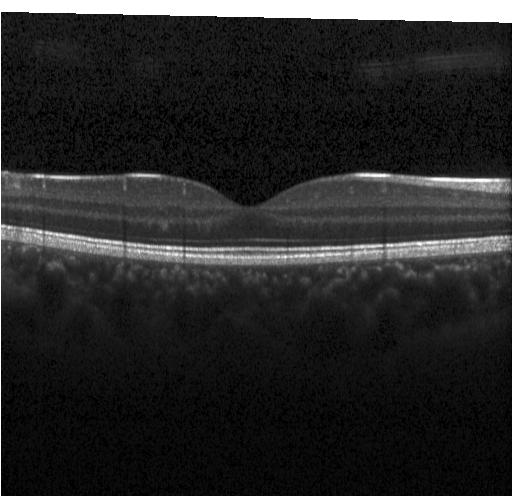

Diagnosis: no evidence of choroidal neovascularization, diabetic macular edema, or drusen.